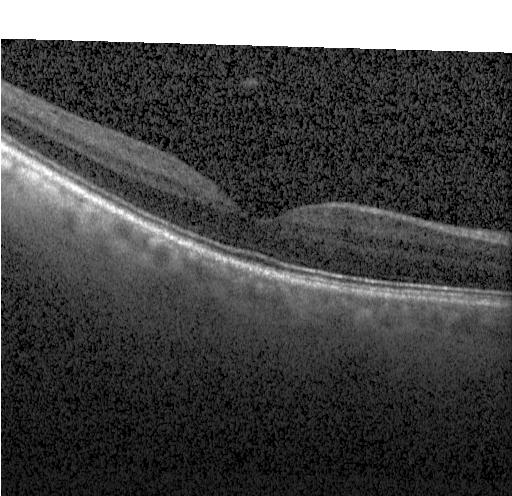 The scan shows no choroidal neovascularization, no diabetic macular edema, and no drusen.